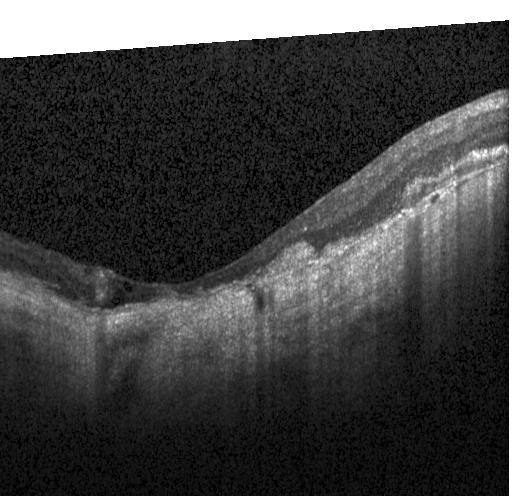 This B-scan demonstrates choroidal neovascularization (CNV).